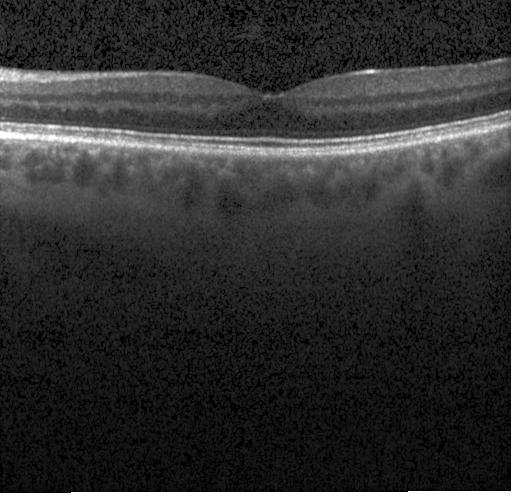 Horizontal scan through the fovea; retinal OCT cross-section; spectral-domain OCT — Impression: no choroidal neovascularization, diabetic macular edema, or drusen.